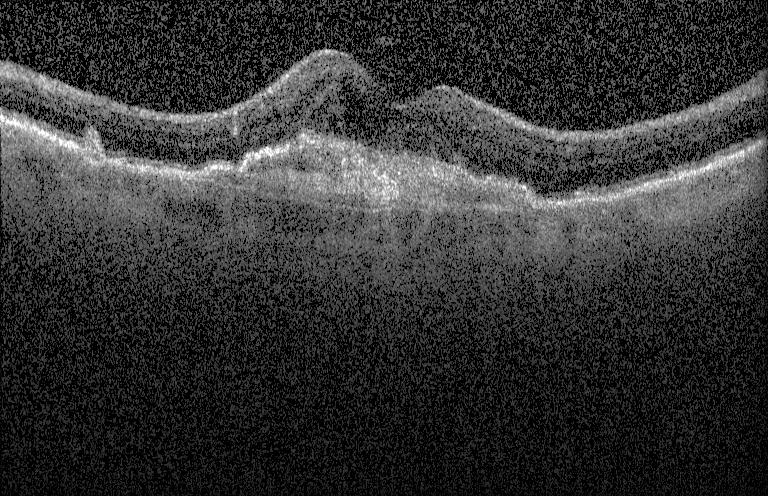
OCT line scan
The scan shows a choroidal neovascular membrane.